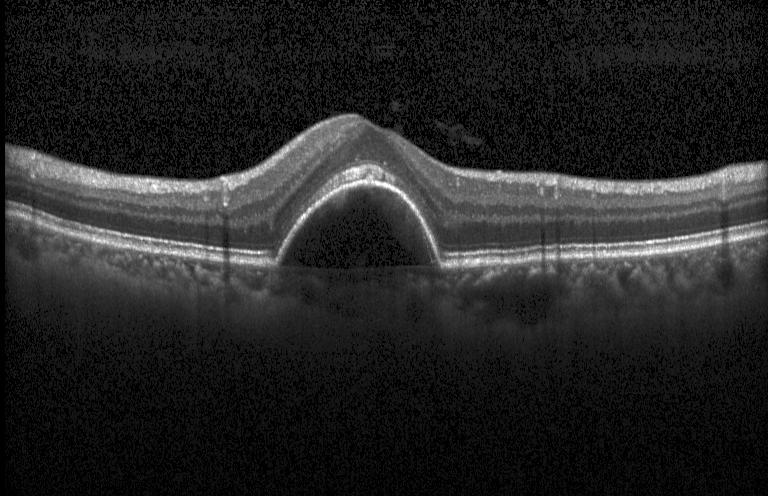
OCT line scan · spectral-domain OCT — Finding: a choroidal neovascular membrane.